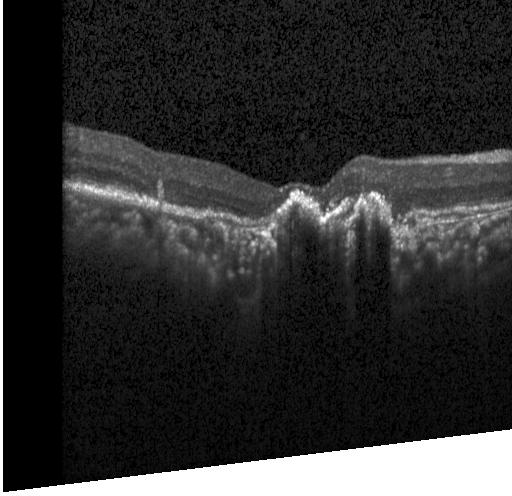

Spectral-domain OCT B-scan: a choroidal neovascular membrane.